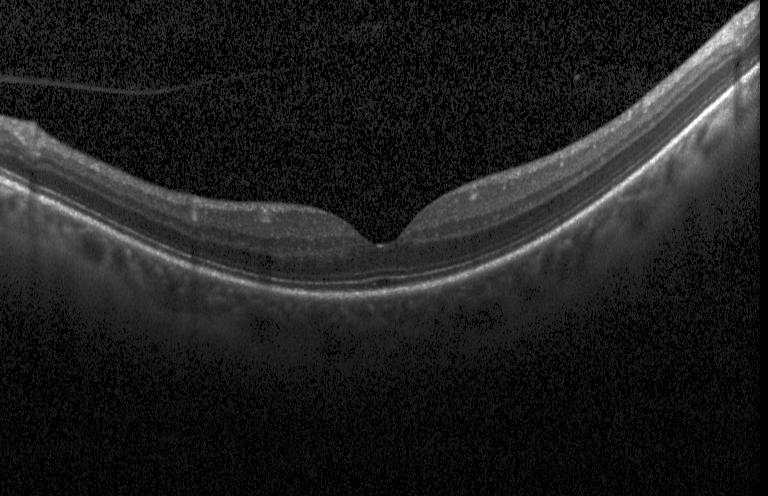
Retinal OCT cross-section
OCT finding: no evidence of choroidal neovascularization, diabetic macular edema, or drusen.